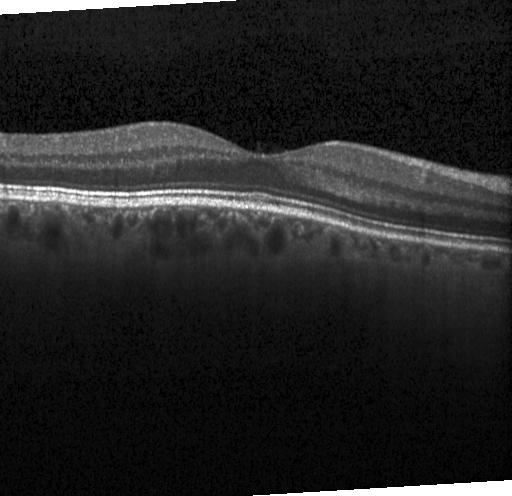 Optical coherence tomography B-scan; centered on the fovea; SD-OCT.
OCT finding: no evidence of choroidal neovascularization, diabetic macular edema, or drusen.